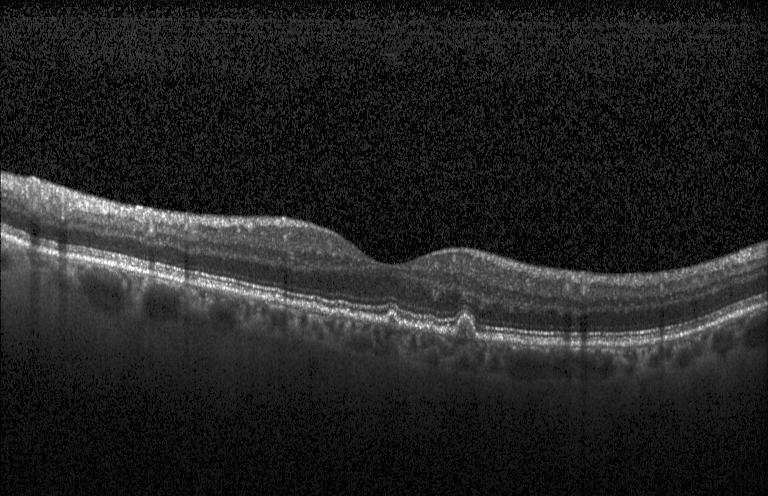 Macular OCT: sub-RPE drusenoid deposits.